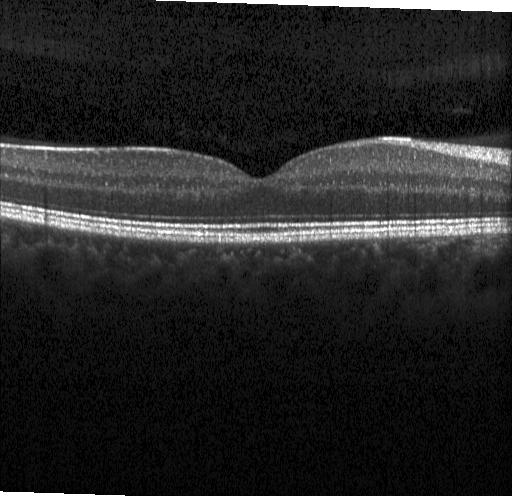
The scan shows no choroidal neovascularization, no diabetic macular edema, and no drusen.